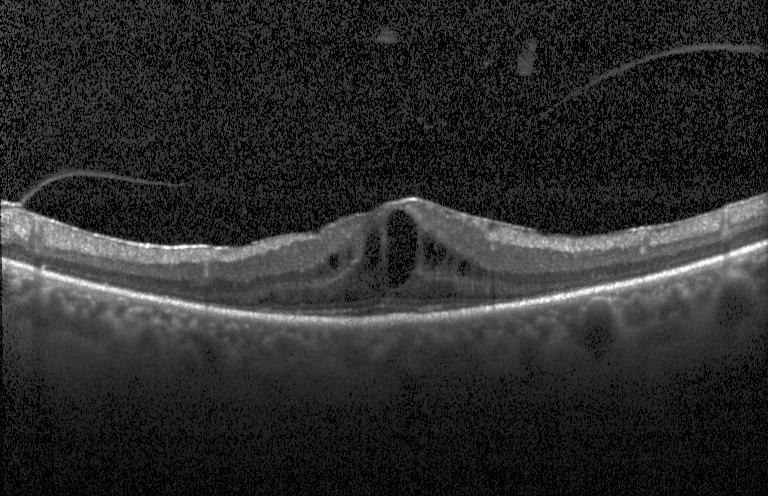 Impression: DME.